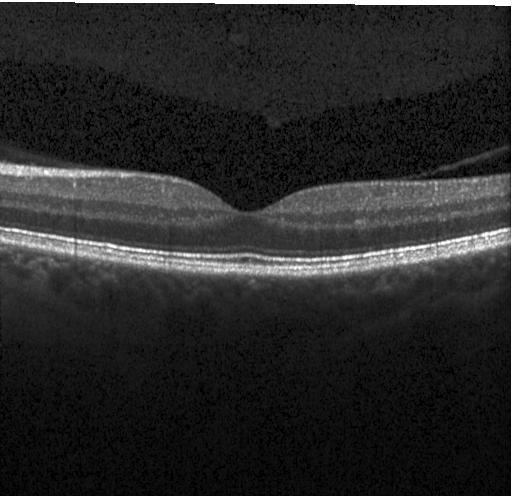 OCT B-scan, through the macula, acquired on a Heidelberg Spectralis, spectral-domain optical coherence tomography.
Macular OCT: neither choroidal neovascularization, diabetic macular edema, nor drusen.